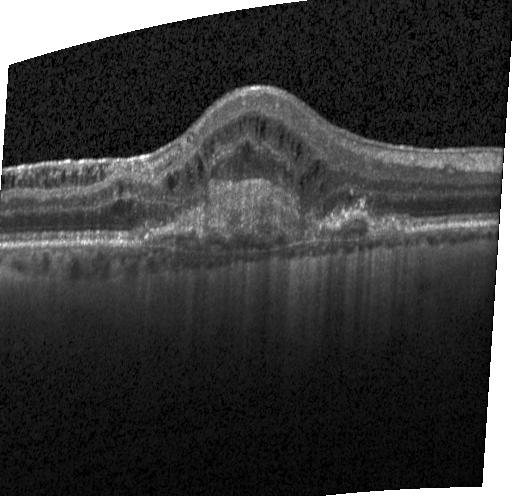
Heidelberg Spectralis OCT system. OCT B-scan — This B-scan demonstrates CNV.